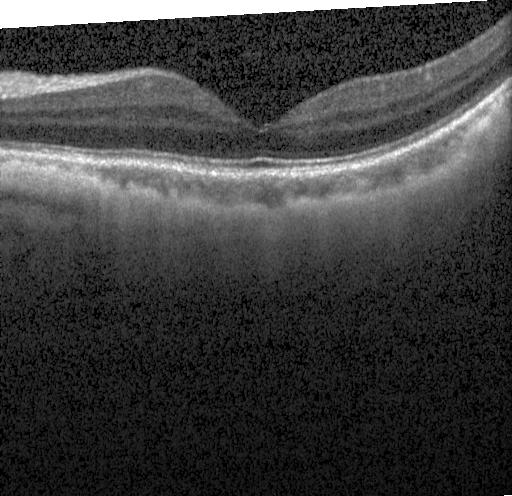

This B-scan demonstrates no evidence of choroidal neovascularization, diabetic macular edema, or drusen.